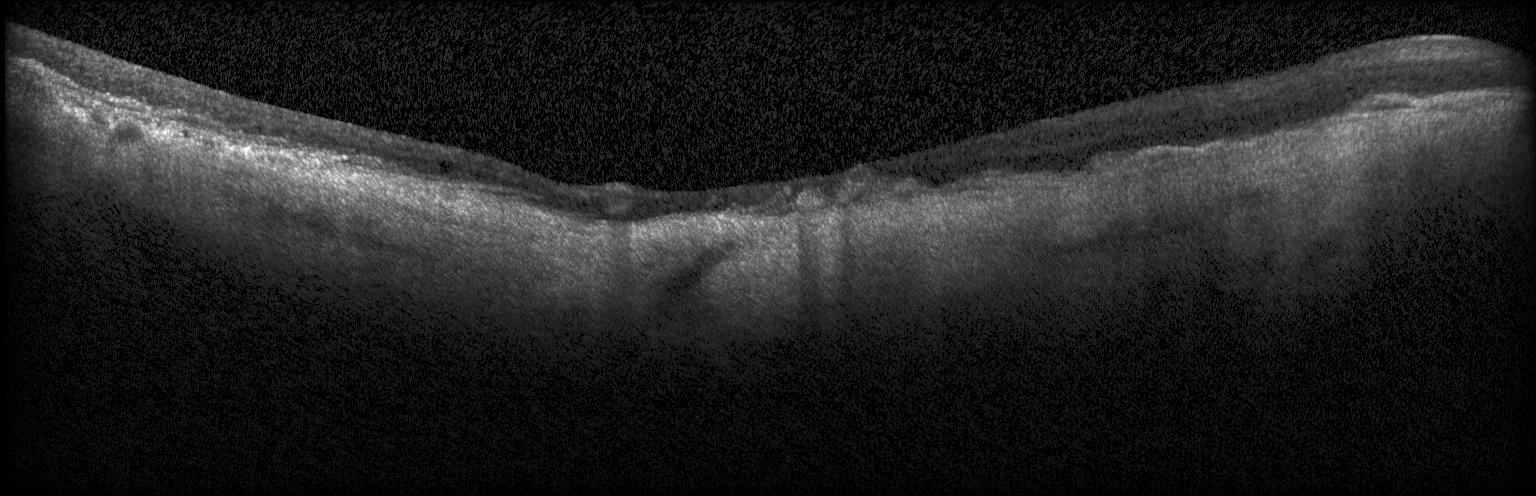
Macular OCT demonstrating CNV.